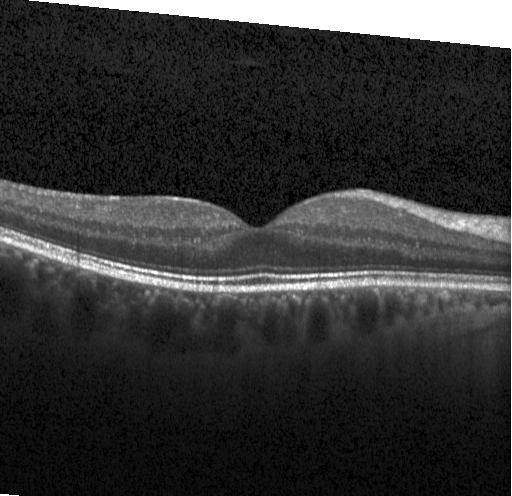
Heidelberg Spectralis OCT system; through the macula; retinal OCT B-scan.
This B-scan demonstrates no choroidal neovascularization, diabetic macular edema, or drusen.